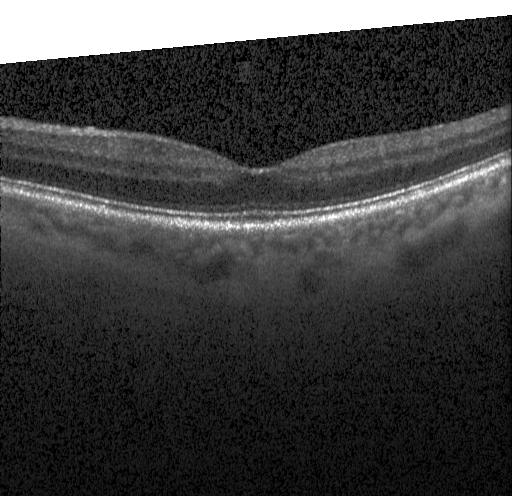

Spectral-domain optical coherence tomography. Optical coherence tomography scan. Heidelberg Spectralis. Finding: no choroidal neovascularization, no diabetic macular edema, and no drusen.